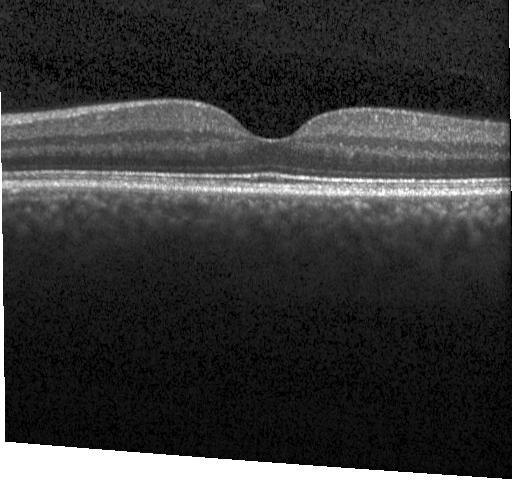

Diagnosis: no choroidal neovascularization, diabetic macular edema, or drusen.